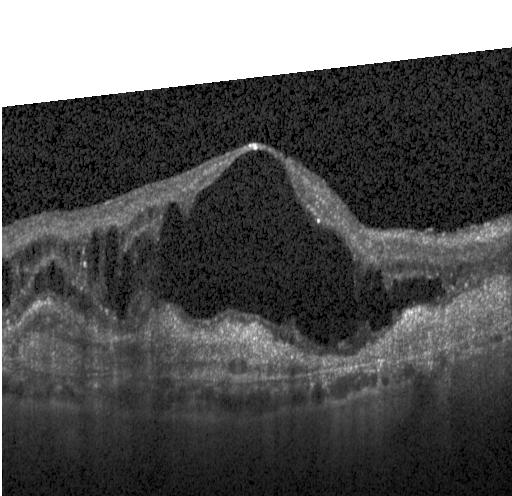
Optical coherence tomography scan.
This B-scan demonstrates a choroidal neovascular membrane.